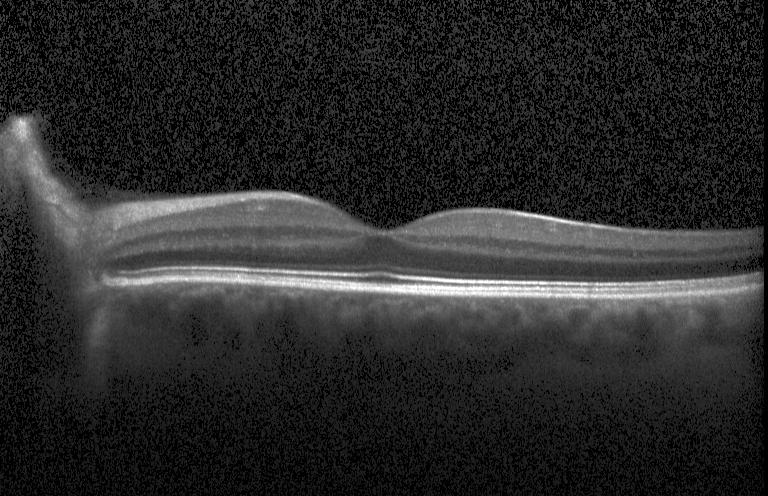
Optical coherence tomography scan. Through the macula.
No choroidal neovascularization, no diabetic macular edema, and no drusen.